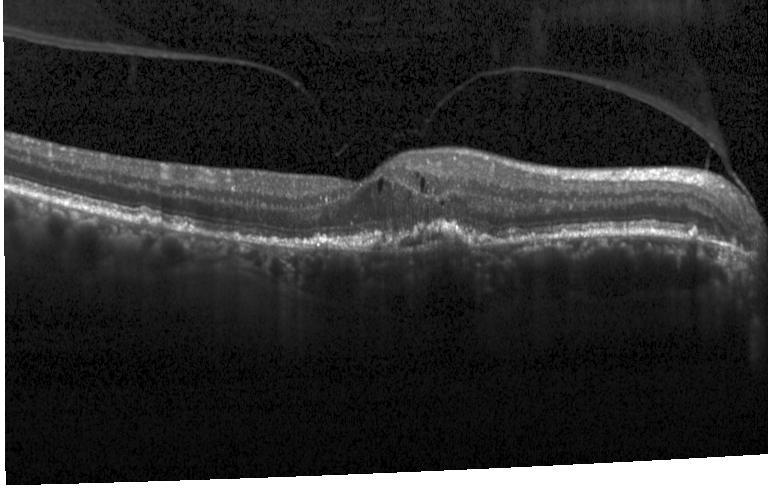 OCT B-scan showing CNV.